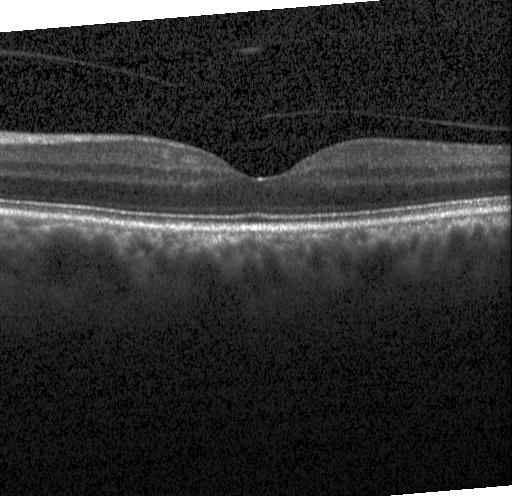

Optical coherence tomography B-scan. Heidelberg Spectralis. SD-OCT. Macular scan.
Impression: neither choroidal neovascularization, diabetic macular edema, nor drusen.